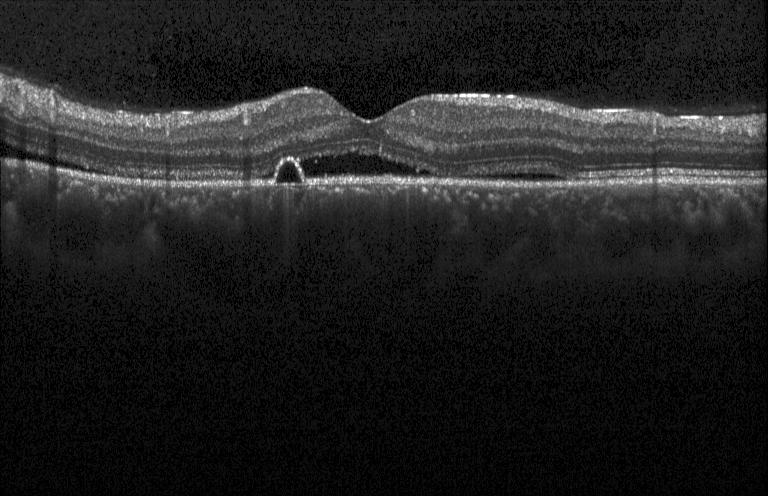
OCT B-scan showing choroidal neovascularization.